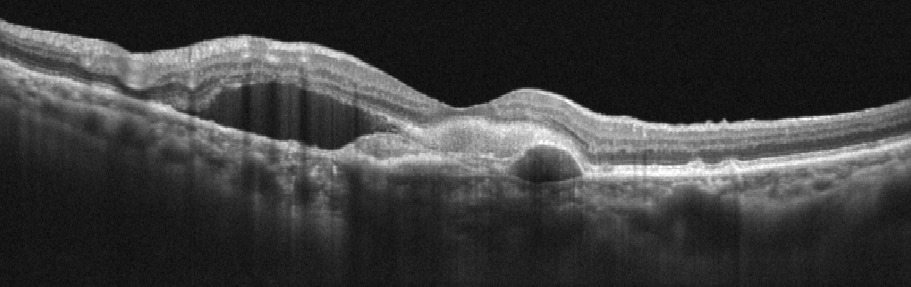
Retinal OCT B-scan — Diagnosis: AMD.